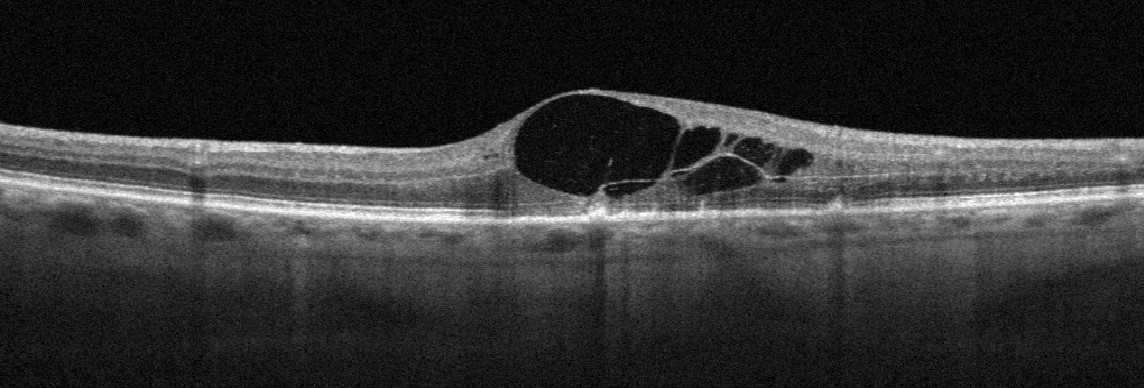

Diagnosis: retinal vein occlusion (RVO).